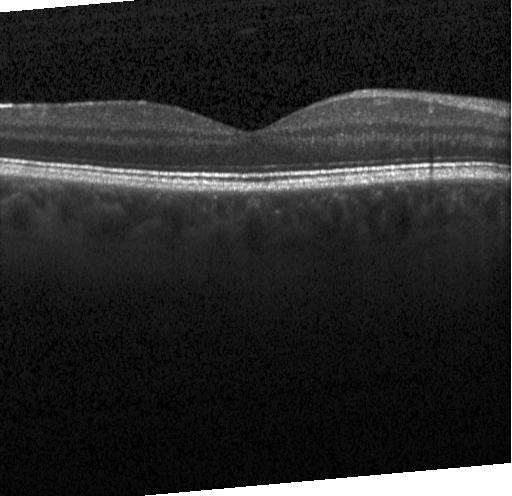
Spectral-domain optical coherence tomography. OCT B-scan. Acquired on a Heidelberg Spectralis
Finding: neither choroidal neovascularization, diabetic macular edema, nor drusen.